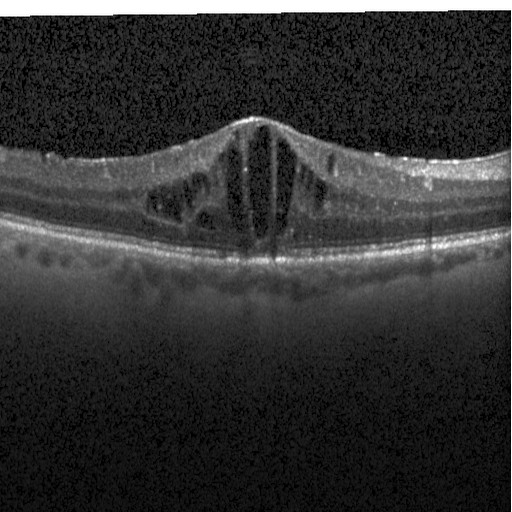 Fovea-centered. Heidelberg Spectralis. Spectral-domain optical coherence tomography. Retinal OCT cross-section
Diagnosis: diabetic macular edema (DME).